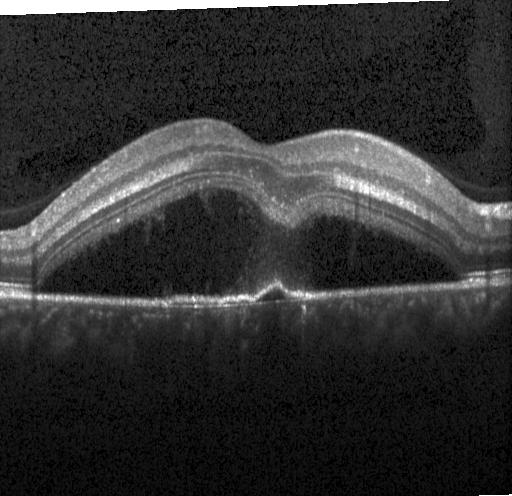

OCT B-scan, Heidelberg Spectralis OCT system — This B-scan demonstrates a choroidal neovascular membrane.